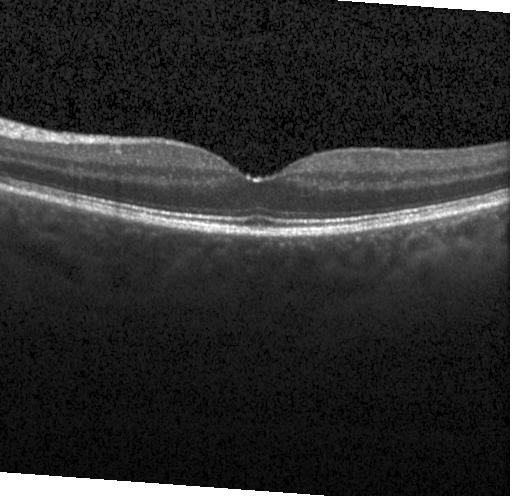
Diagnosis: no choroidal neovascularization, diabetic macular edema, or drusen.